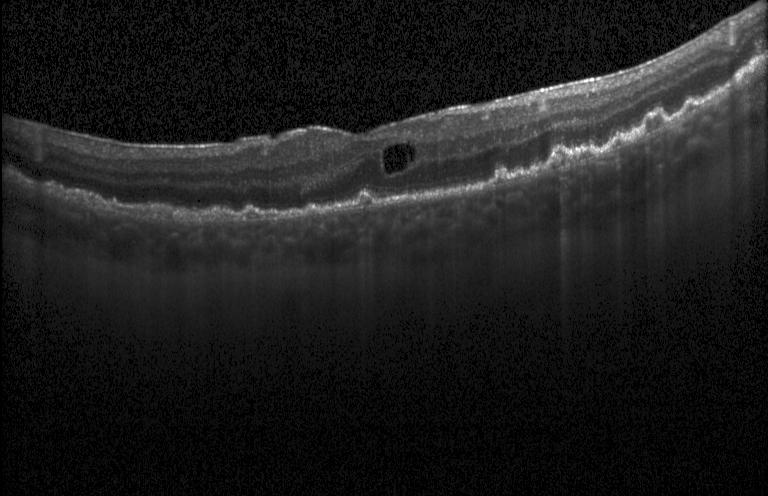
Retinal OCT B-scan · through the macula. Assessment: a choroidal neovascular membrane.